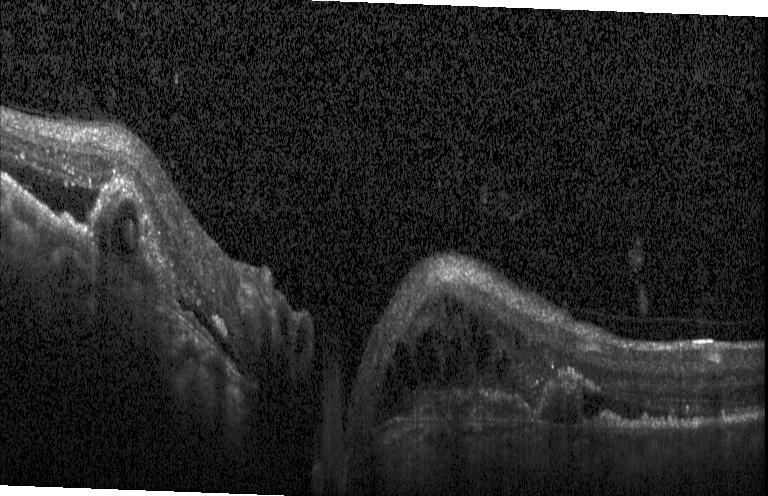 Spectral-domain optical coherence tomography, acquired on a Heidelberg Spectralis, through the macula, retinal OCT B-scan — Macular OCT: CNV.